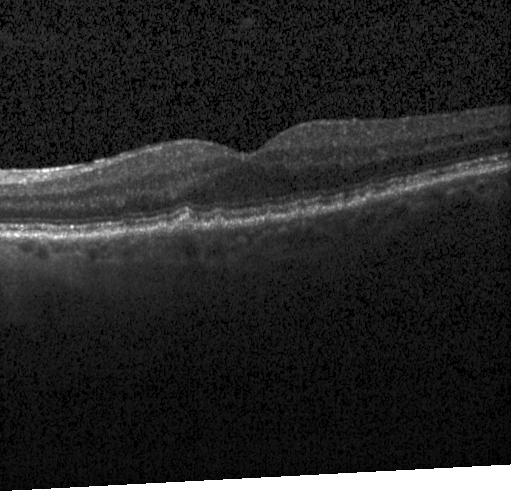

Optical coherence tomography scan
Diagnosis: sub-RPE drusenoid deposits.